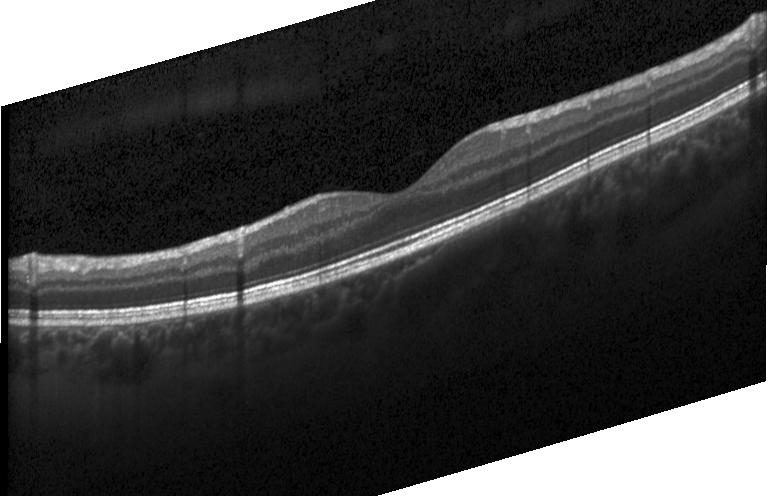
Heidelberg Spectralis OCT system, retinal OCT cross-section, SD-OCT.
Diagnosis: no CNV, no DME, and no drusen.